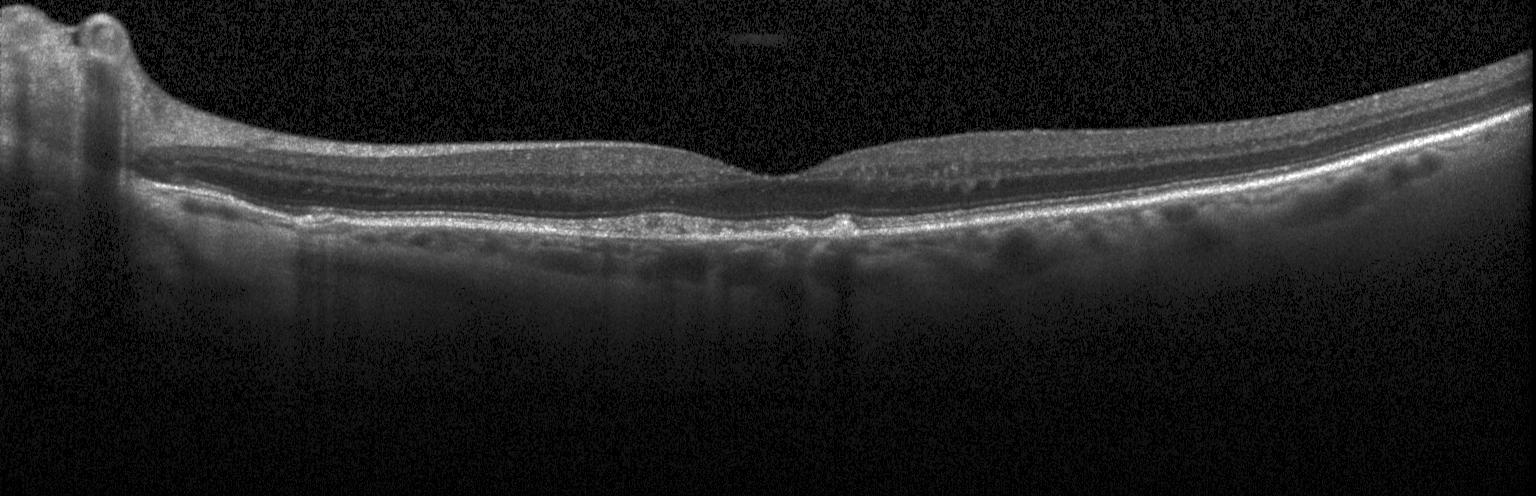

Optical coherence tomography scan.
Finding: multiple drusen.